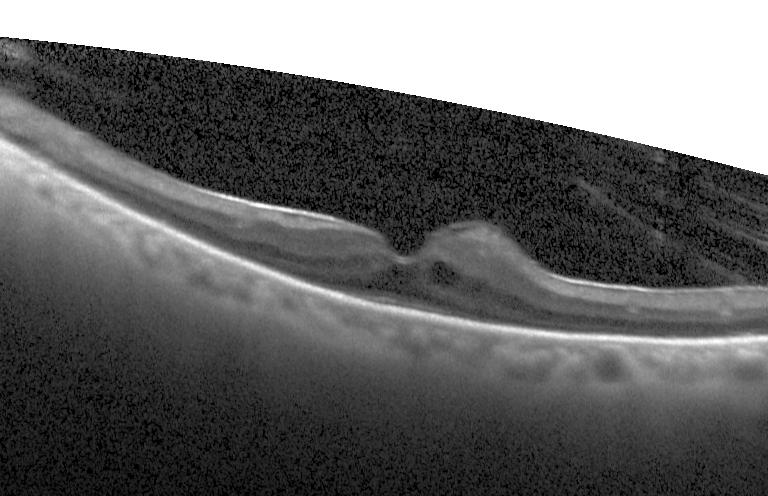

Retinal OCT cross-section. Macular OCT: DME.